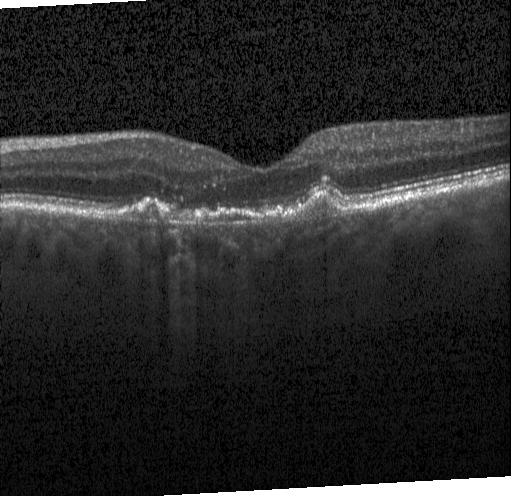 Spectral-domain OCT B-scan: a choroidal neovascular membrane.